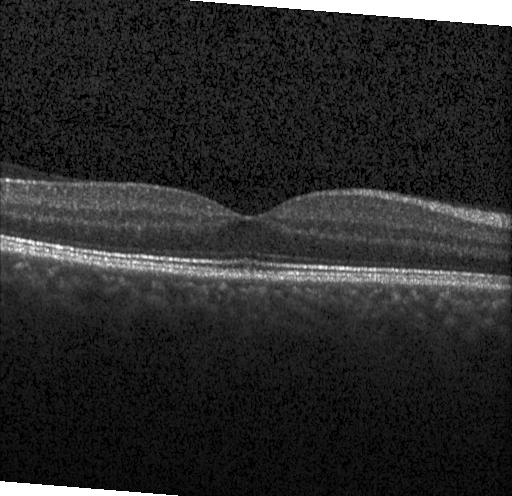

Retinal OCT B-scan; Heidelberg Spectralis — Impression: no CNV, DME, or drusen.